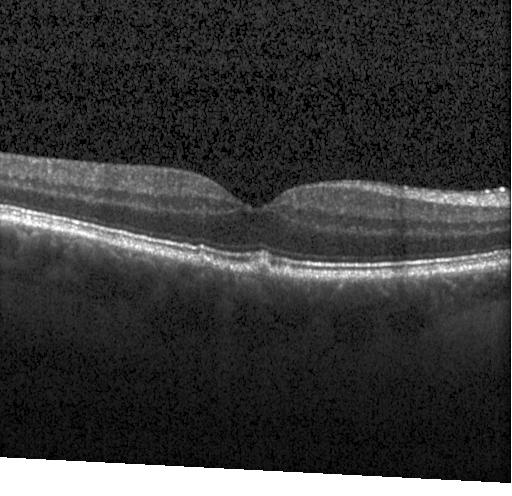 OCT B-scan showing sub-RPE drusenoid deposits.